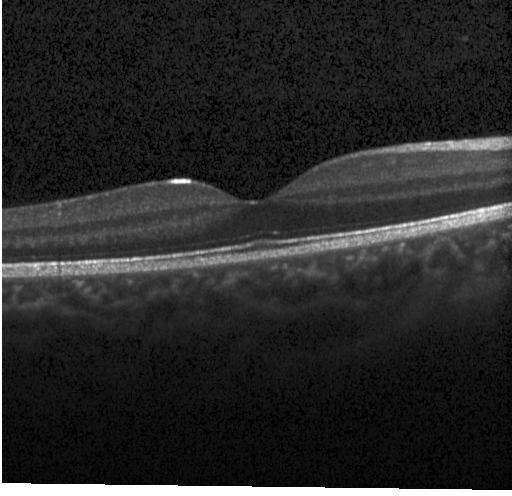

Optical coherence tomography scan.
Neither CNV, DME, nor drusen.